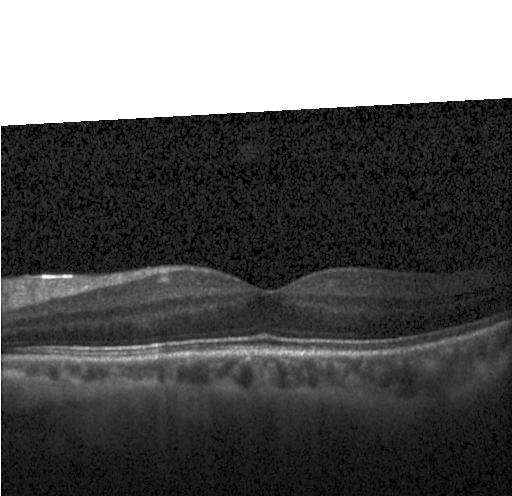
Optical coherence tomography scan — The scan shows neither choroidal neovascularization, diabetic macular edema, nor drusen.